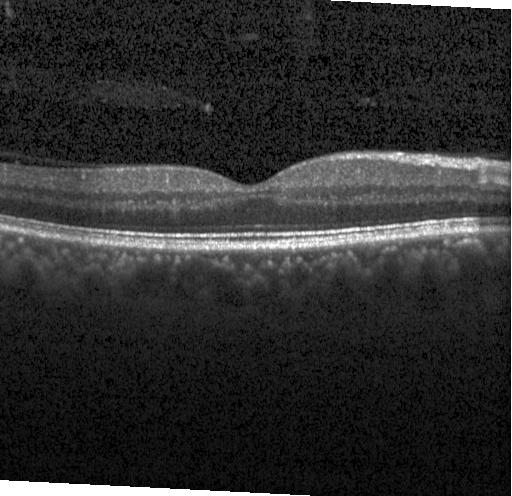

Macular scan, Heidelberg Spectralis OCT system, OCT B-scan, spectral-domain optical coherence tomography. Diagnosis: no evidence of CNV, DME, or drusen.